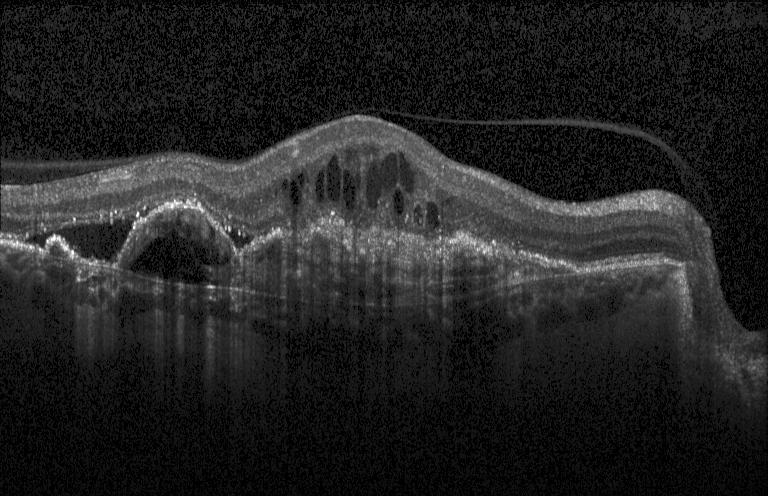

Retinal OCT cross-section · acquired on a Heidelberg Spectralis. Impression: a choroidal neovascular membrane.